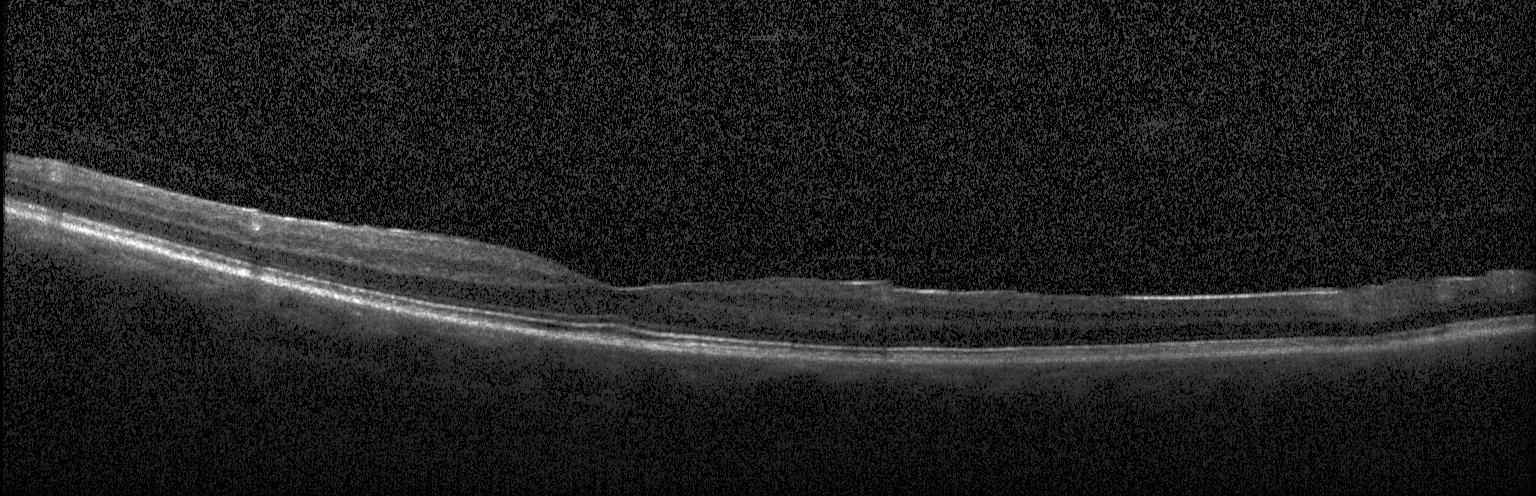

Retinal OCT B-scan — OCT finding: no choroidal neovascularization, no diabetic macular edema, and no drusen.